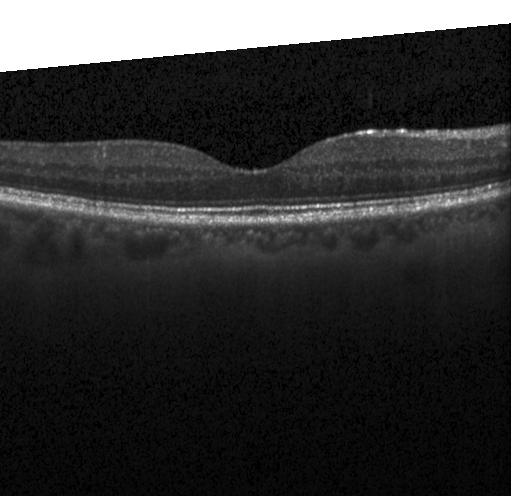

Spectral-domain OCT, centered on the fovea, optical coherence tomography B-scan, Heidelberg Spectralis OCT system. No choroidal neovascularization, diabetic macular edema, or drusen.